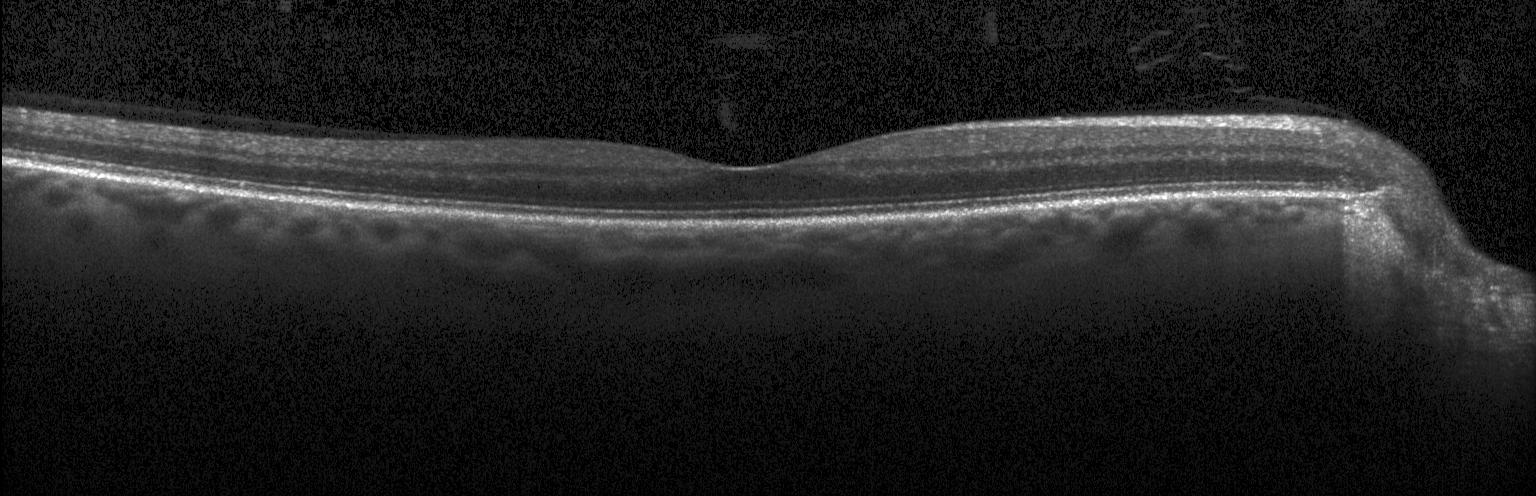

Spectral-domain OCT · OCT B-scan · Heidelberg Spectralis.
Finding: no CNV, no DME, and no drusen.